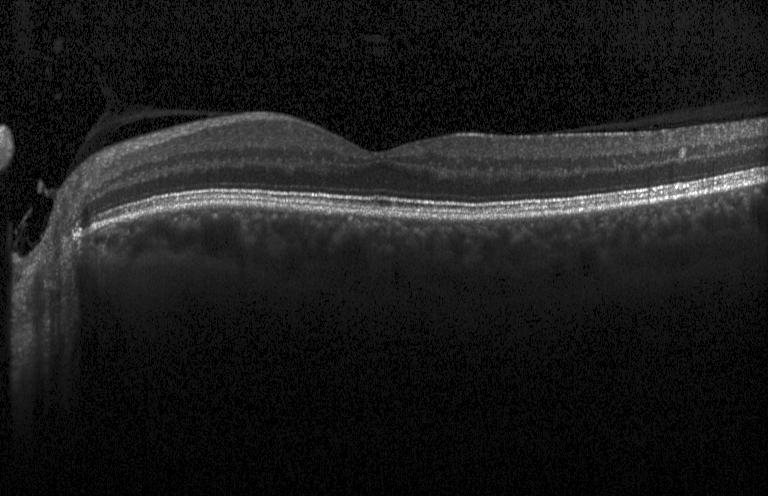

Heidelberg Spectralis, retinal OCT B-scan. Dx: no evidence of choroidal neovascularization, diabetic macular edema, or drusen.